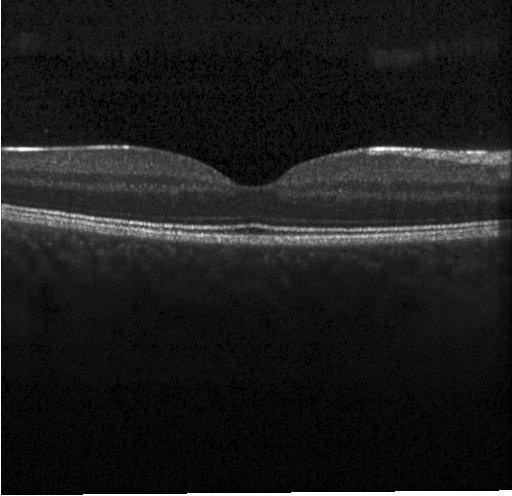

Heidelberg Spectralis OCT system, SD-OCT, OCT line scan.
Diagnosis: no choroidal neovascularization, diabetic macular edema, or drusen.